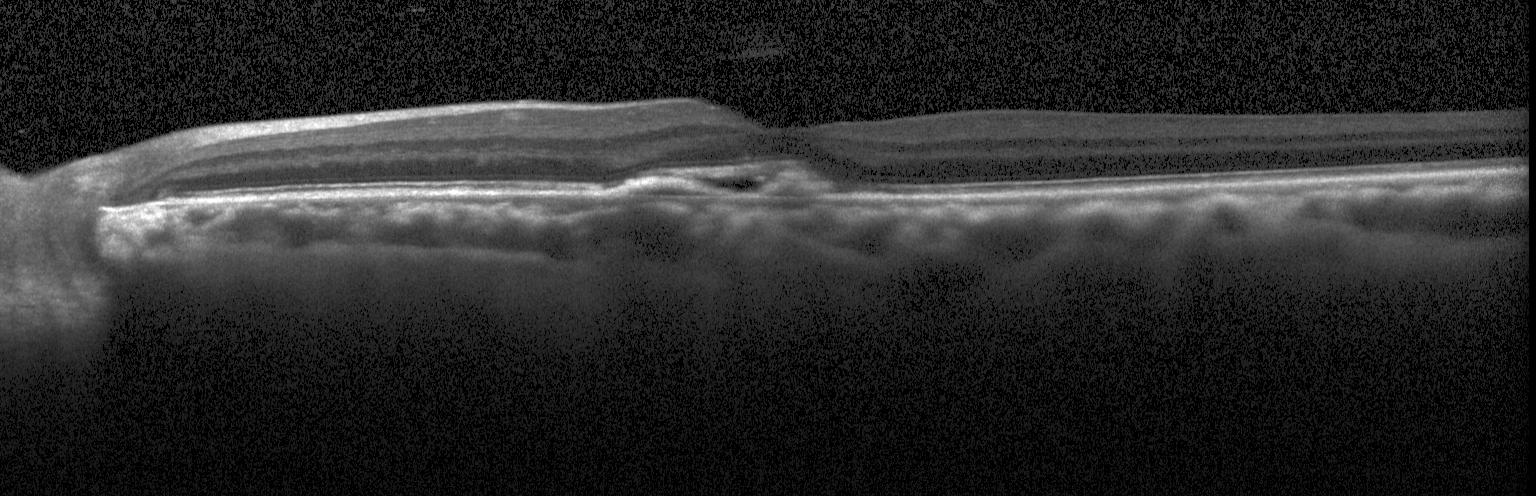 Spectral-domain OCT B-scan: a choroidal neovascular membrane.